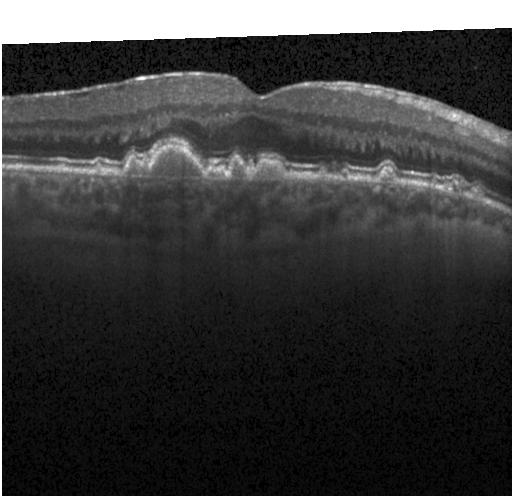
OCT B-scan. Spectral-domain optical coherence tomography. Heidelberg Spectralis. Horizontal scan through the fovea. This B-scan demonstrates a choroidal neovascular membrane.